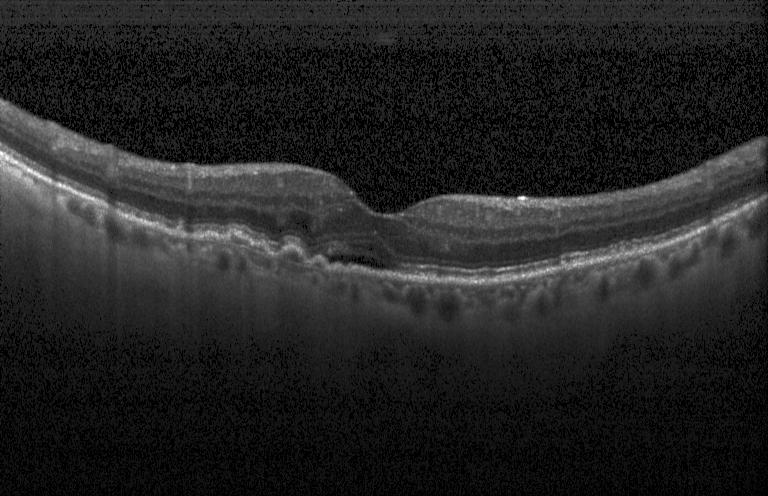 Through the macula · Heidelberg Spectralis OCT system · SD-OCT · OCT B-scan.
Dx: a choroidal neovascular membrane.